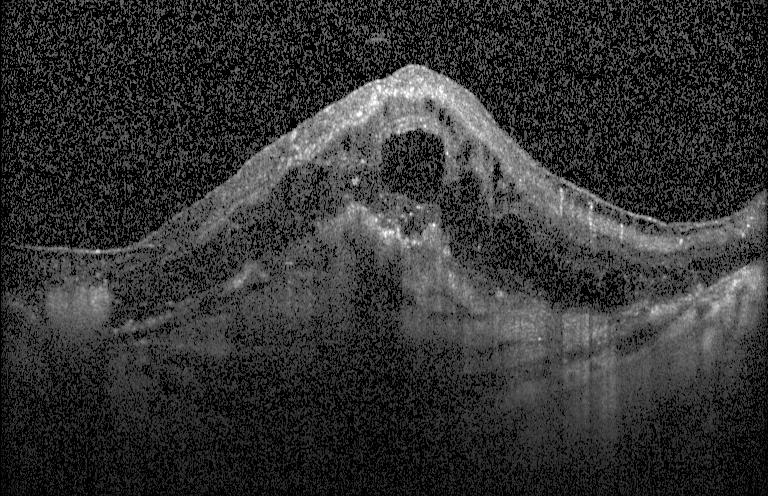 OCT B-scan · instrument: Heidelberg Spectralis. Assessment: CNV.